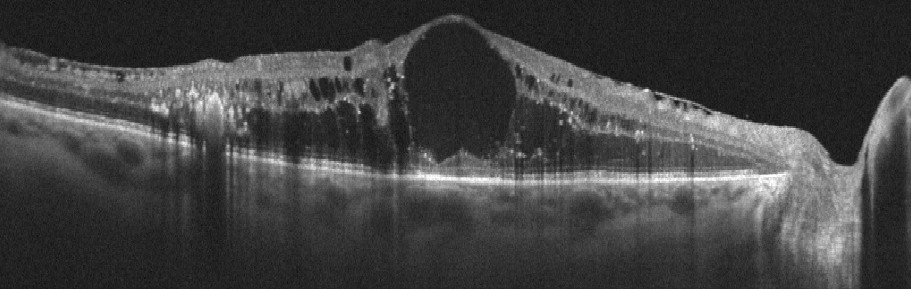 Dx: diabetic macular edema.